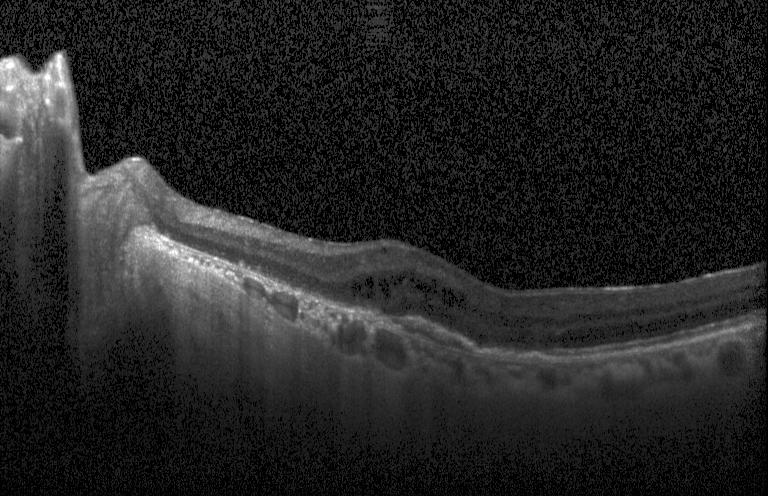

Retinal OCT cross-section.
This B-scan demonstrates a choroidal neovascular membrane.